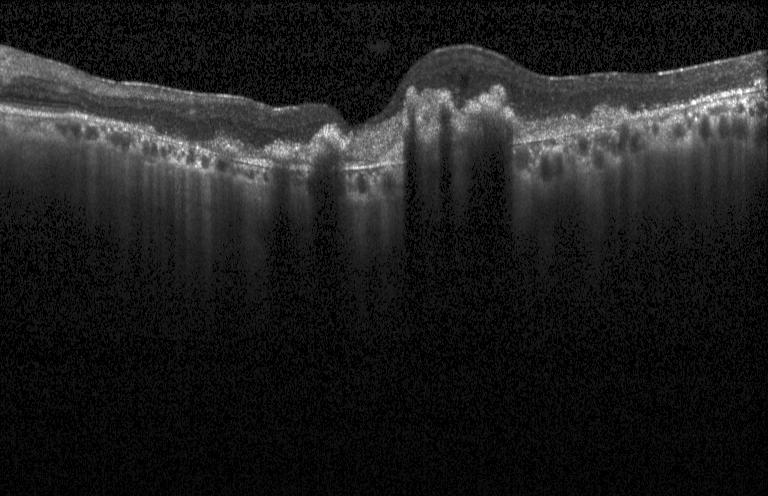
Acquired on a Heidelberg Spectralis · optical coherence tomography scan · fovea-centered
The scan shows a choroidal neovascular membrane.